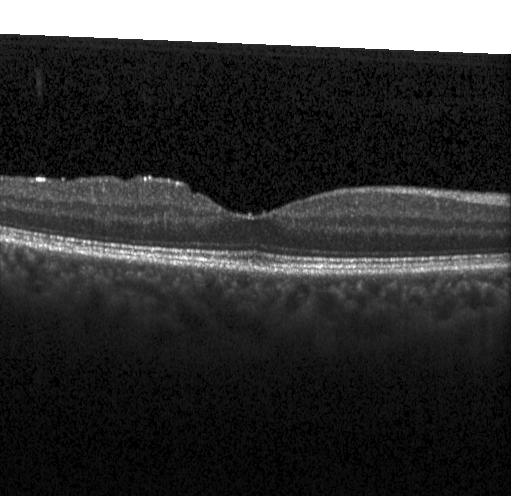
The scan shows no evidence of choroidal neovascularization, diabetic macular edema, or drusen.